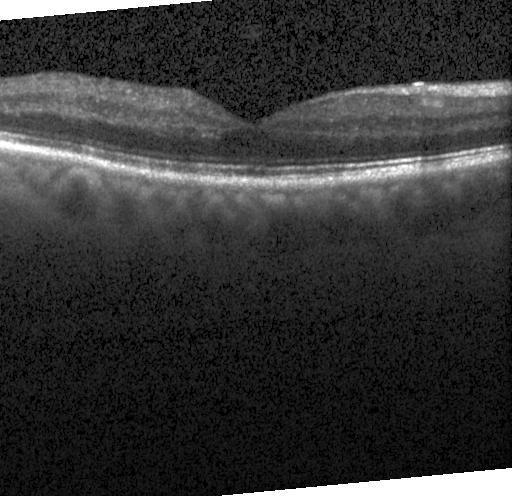 This B-scan demonstrates no choroidal neovascularization, diabetic macular edema, or drusen.